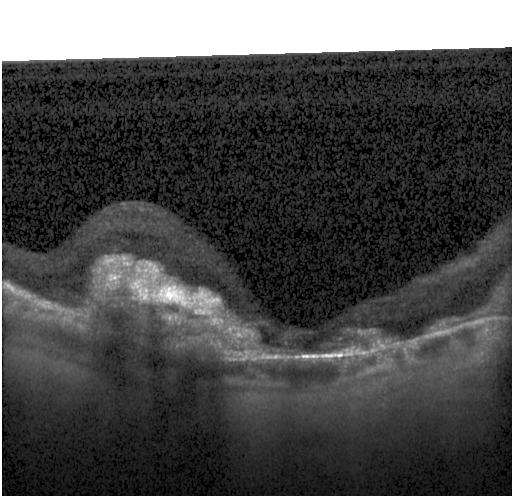
Optical coherence tomography scan
OCT finding: choroidal neovascularization.